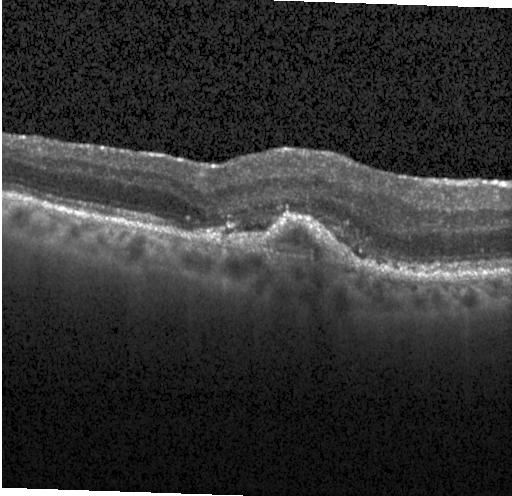

Finding: choroidal neovascularization (CNV).